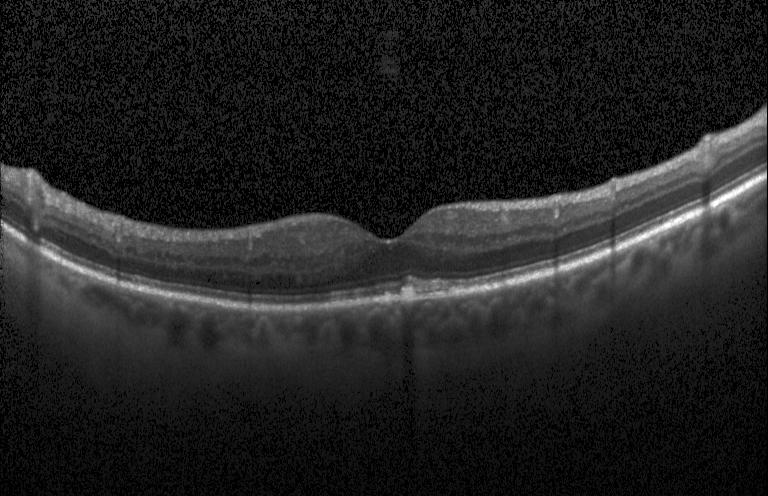
Retinal OCT B-scan.
The scan shows sub-RPE drusenoid deposits.